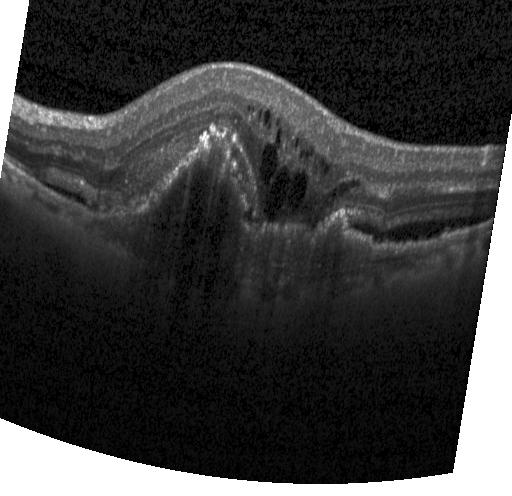 Spectral-domain optical coherence tomography · optical coherence tomography B-scan — Diagnosis: CNV.